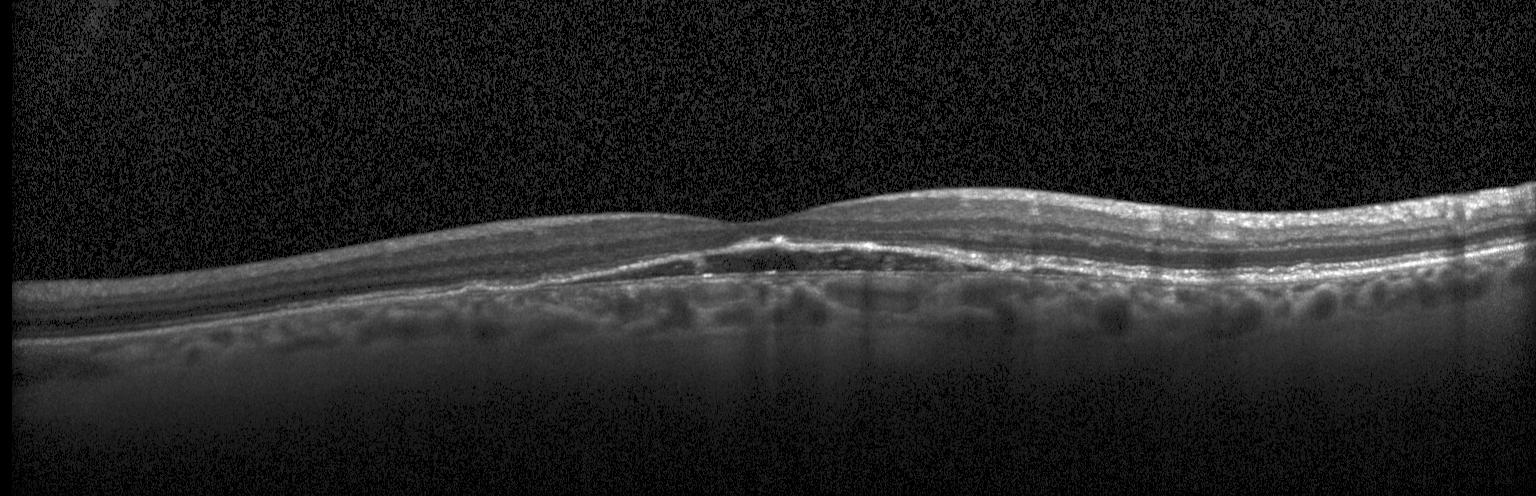 Retinal OCT cross-section
This B-scan demonstrates a choroidal neovascular membrane.